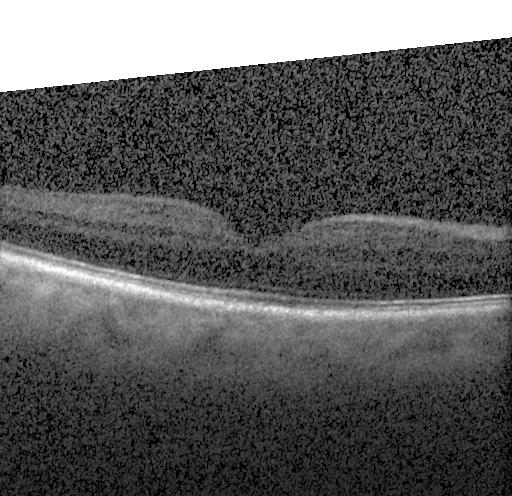 Diagnosis: no CNV, no DME, and no drusen.